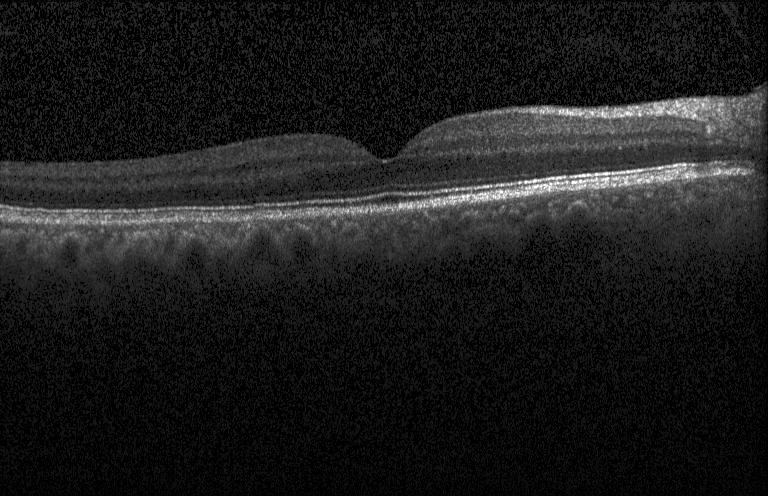
Macular OCT demonstrating no choroidal neovascularization, no diabetic macular edema, and no drusen.